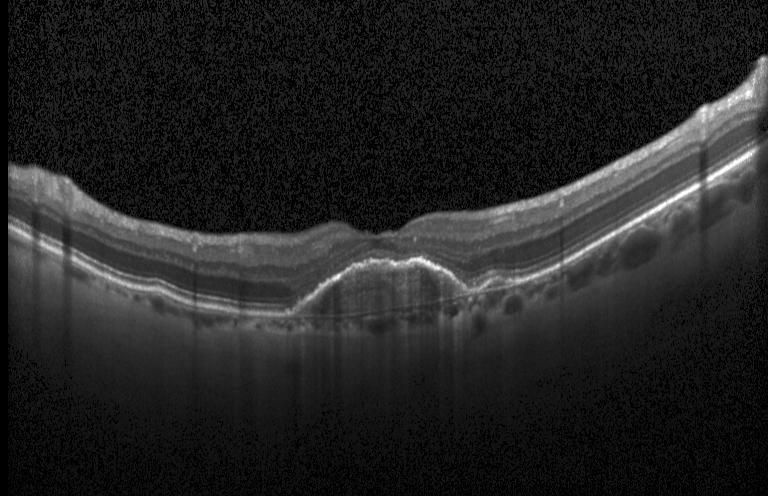
Retinal OCT cross-section showing choroidal neovascularization.